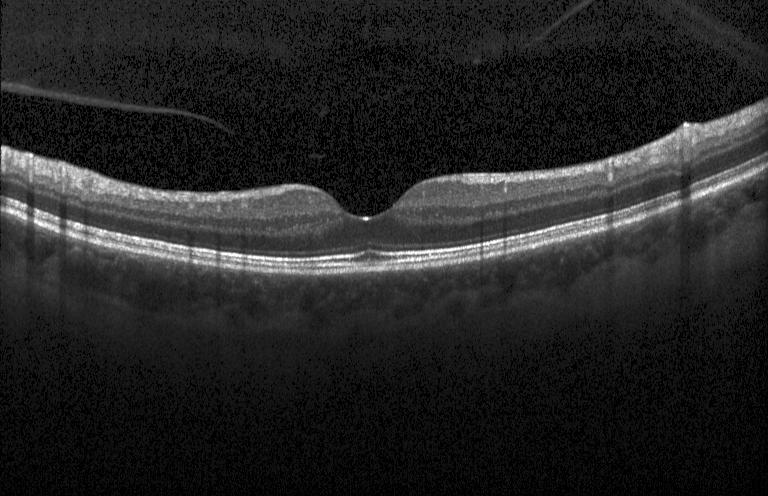

This B-scan demonstrates neither choroidal neovascularization, diabetic macular edema, nor drusen.